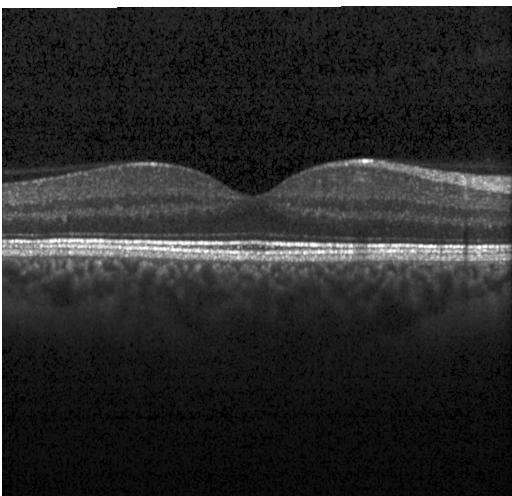

Impression: neither choroidal neovascularization, diabetic macular edema, nor drusen.